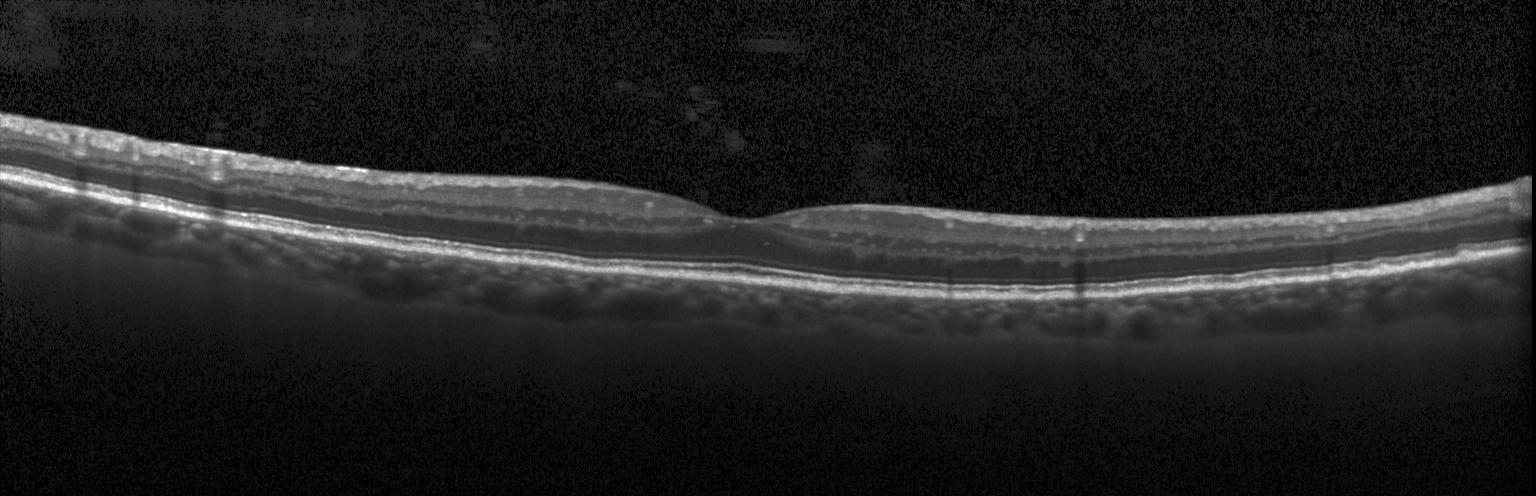
Spectral-domain optical coherence tomography, through the macula, optical coherence tomography scan, Heidelberg Spectralis. Finding: no choroidal neovascularization, diabetic macular edema, or drusen.